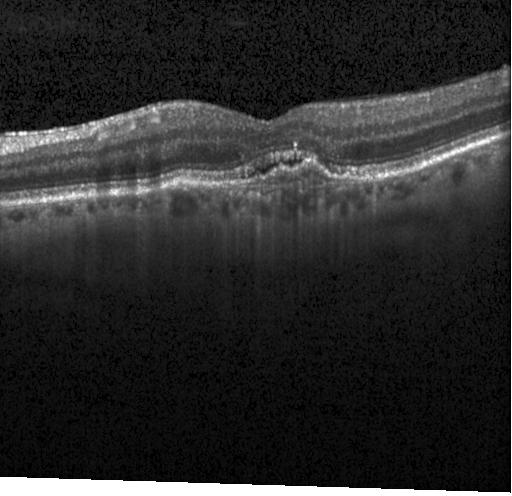

Instrument: Heidelberg Spectralis · centered on the fovea · OCT line scan.
Assessment: choroidal neovascularization.